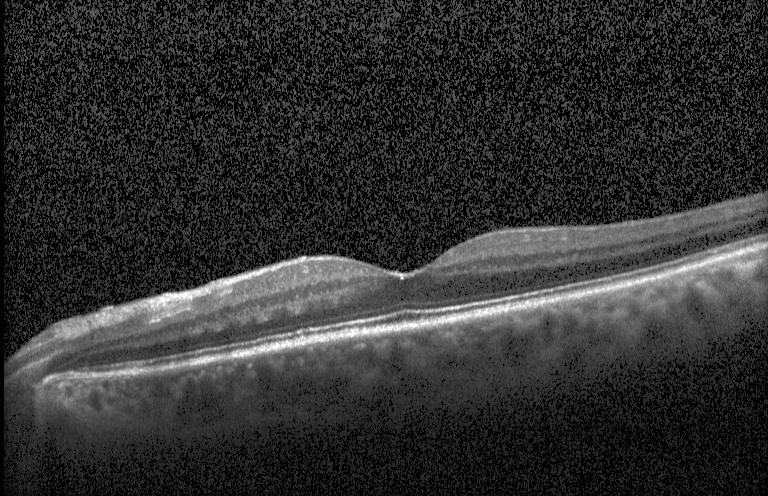
OCT B-scan showing no evidence of choroidal neovascularization, diabetic macular edema, or drusen.